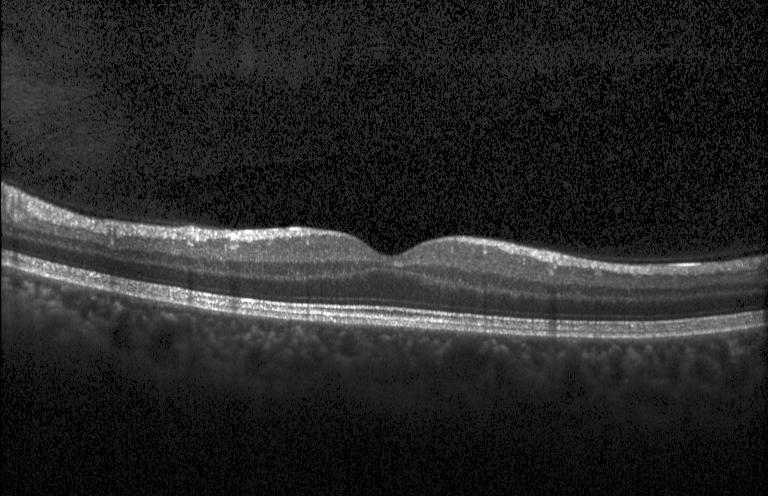 OCT finding: no evidence of choroidal neovascularization, diabetic macular edema, or drusen.